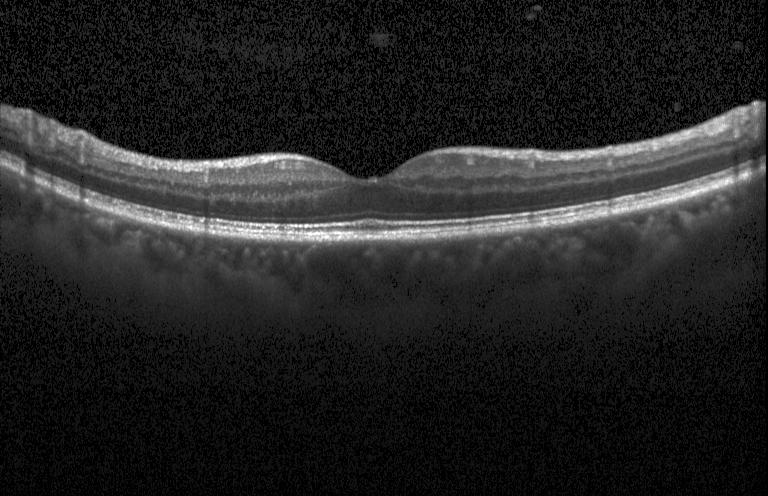 Impression: neither choroidal neovascularization, diabetic macular edema, nor drusen.